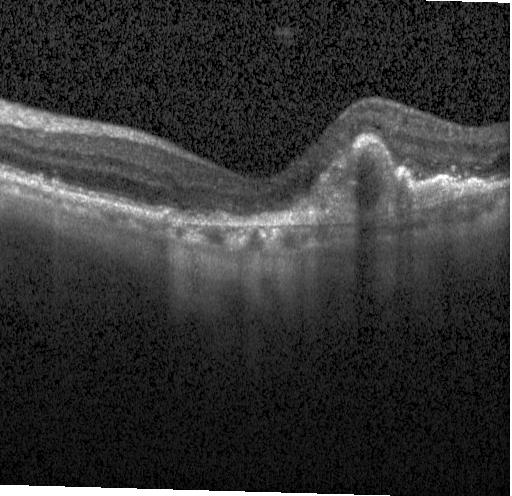

Assessment: a choroidal neovascular membrane.